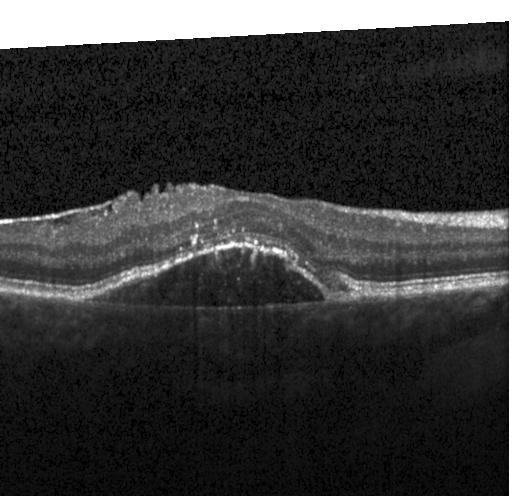
Spectral-domain optical coherence tomography. Through the macula. OCT B-scan. Acquired on a Heidelberg Spectralis — A choroidal neovascular membrane.